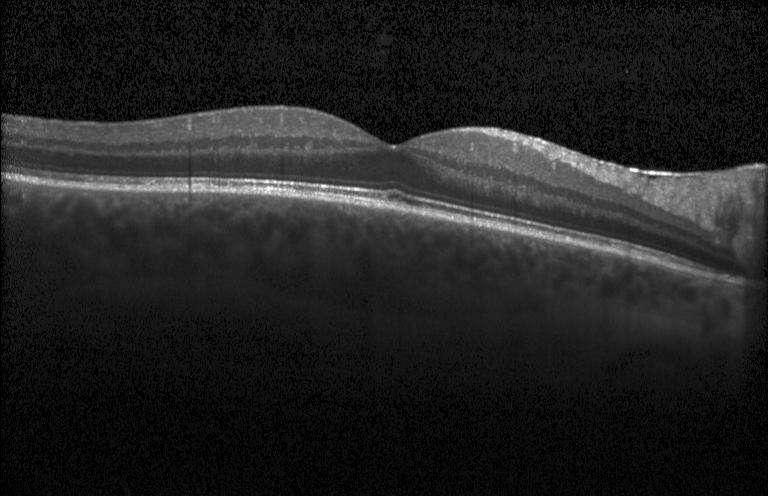 OCT B-scan. No evidence of CNV, DME, or drusen.